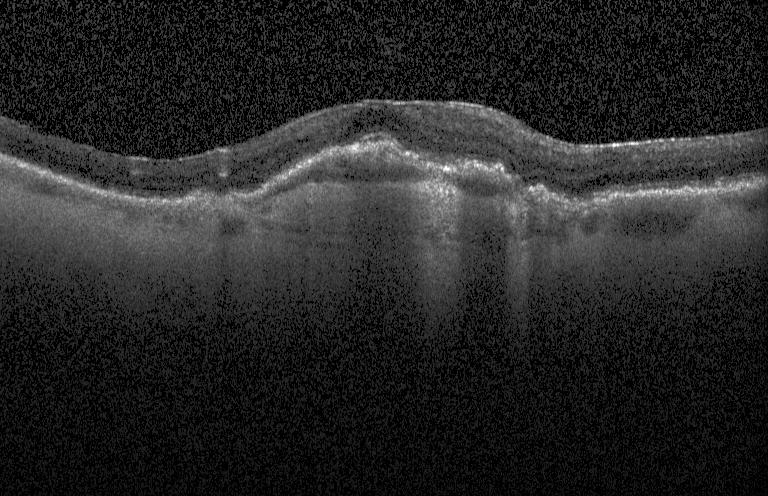
Macular OCT demonstrating a choroidal neovascular membrane.